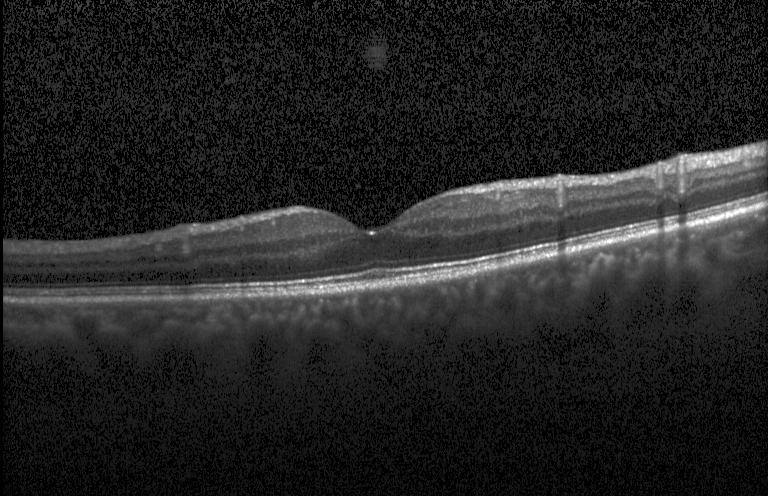 SD-OCT · horizontal scan through the fovea · optical coherence tomography B-scan. No choroidal neovascularization, no diabetic macular edema, and no drusen.